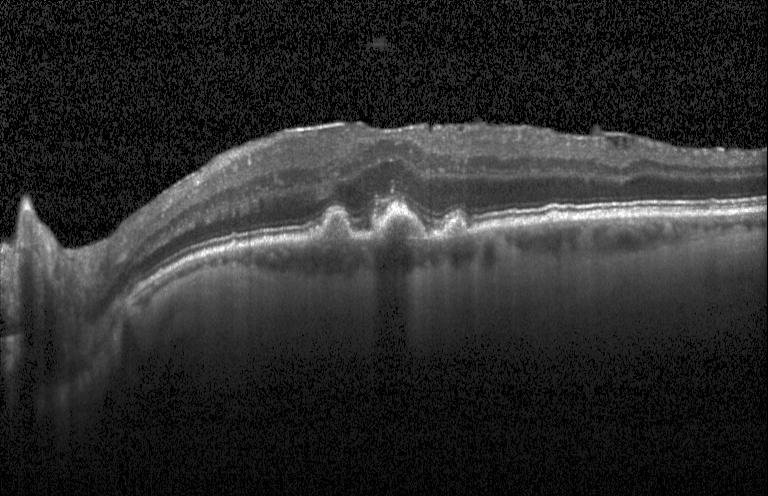

Impression: sub-RPE drusenoid deposits.